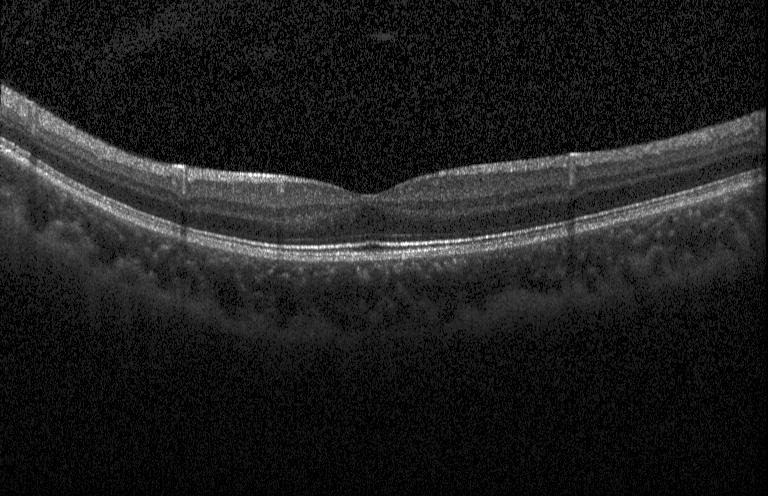

Retinal OCT B-scan; macular scan; SD-OCT; Heidelberg Spectralis OCT system — Diagnosis: neither CNV, DME, nor drusen.